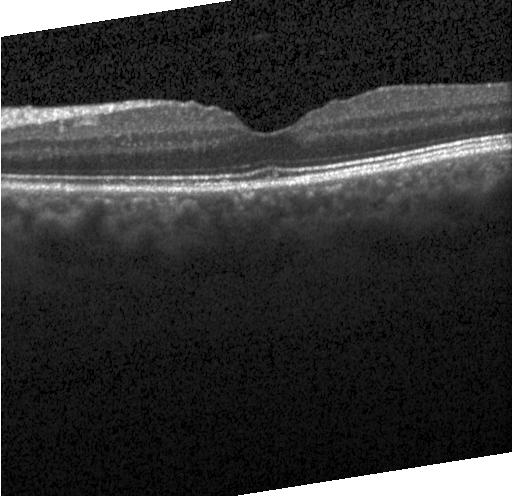 No choroidal neovascularization, diabetic macular edema, or drusen.